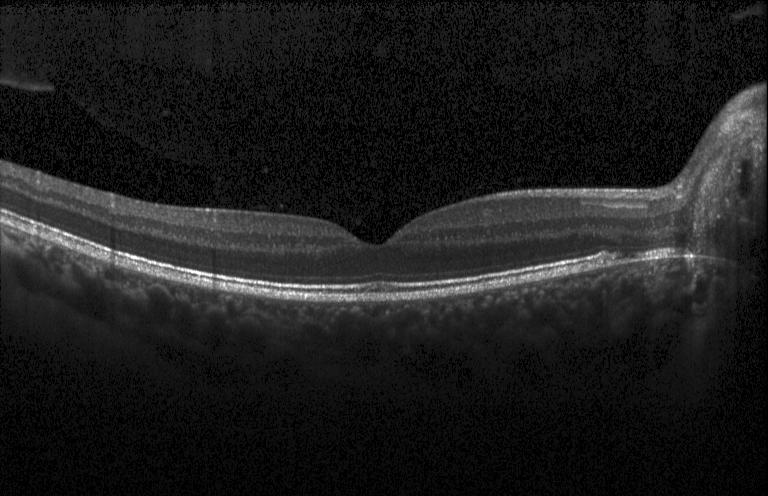
OCT line scan. Fovea-centered. Acquired on a Heidelberg Spectralis — Diagnosis: no evidence of choroidal neovascularization, diabetic macular edema, or drusen.